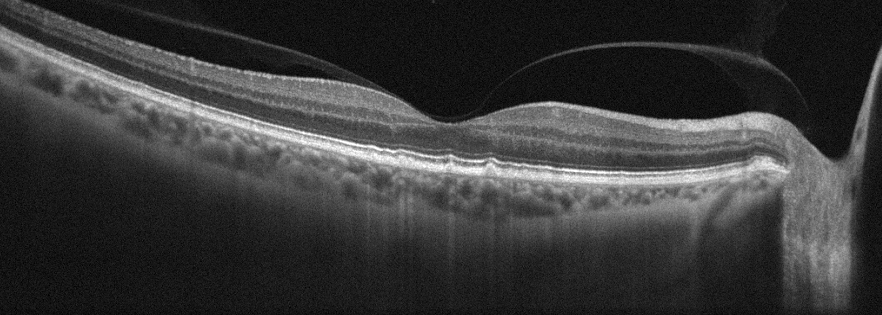

Optical coherence tomography B-scan.
The scan shows age-related macular degeneration (AMD).